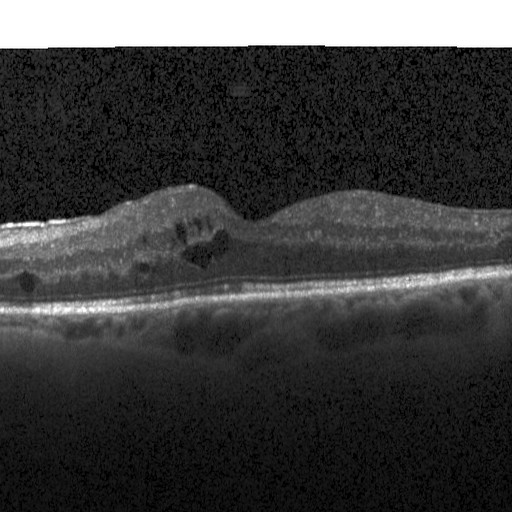
Spectral-domain optical coherence tomography, optical coherence tomography B-scan, fovea-centered, Heidelberg Spectralis OCT system
The scan shows DME.